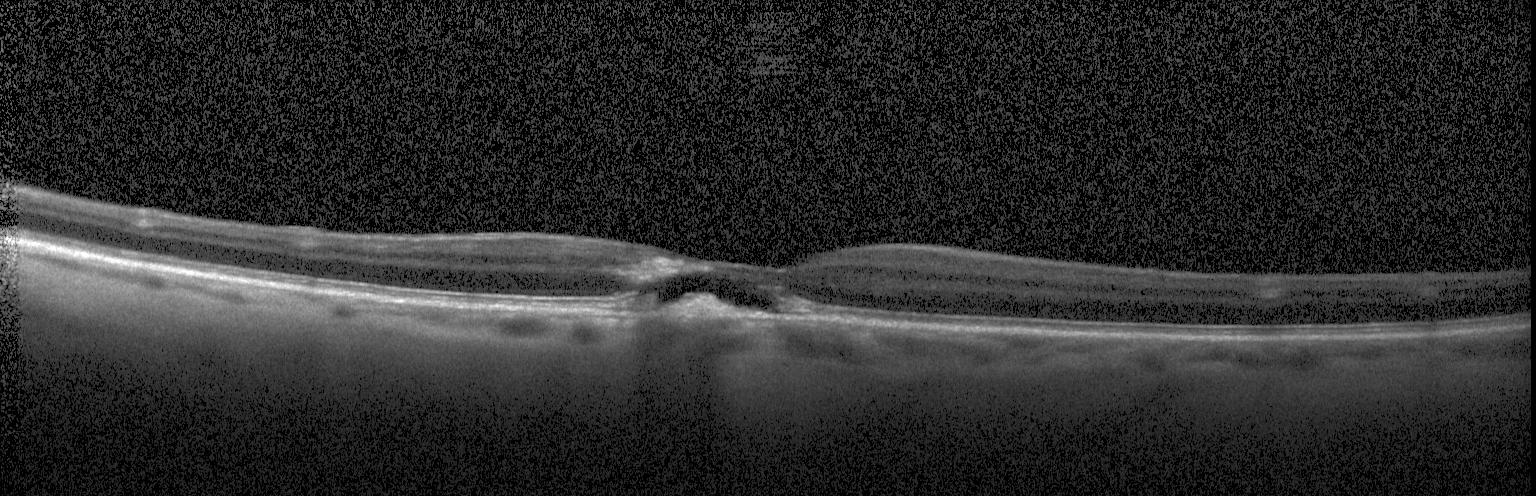
Finding: CNV.